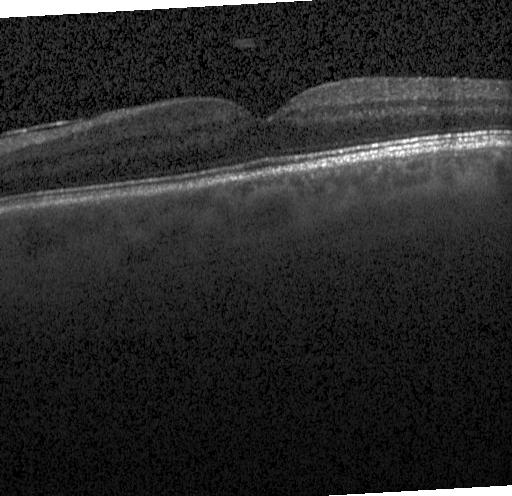

OCT line scan — Dx: no choroidal neovascularization, no diabetic macular edema, and no drusen.